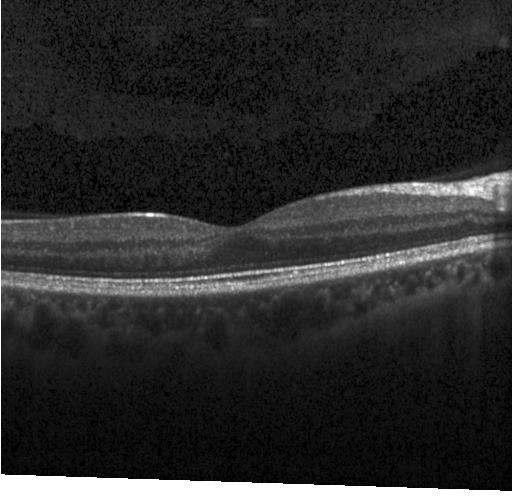

Macular OCT: neither choroidal neovascularization, diabetic macular edema, nor drusen.